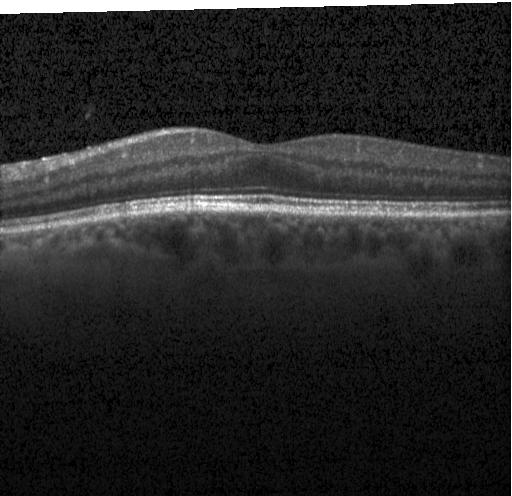
Spectral-domain OCT; fovea-centered; retinal OCT cross-section
Impression: no choroidal neovascularization, no diabetic macular edema, and no drusen.